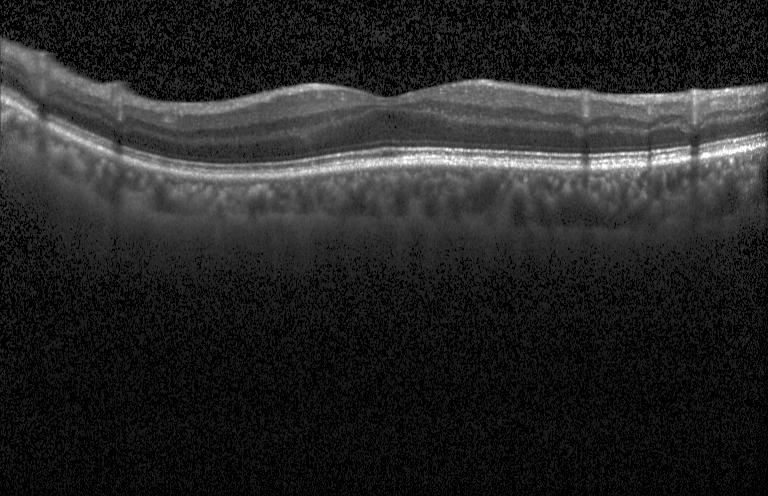

Dx: neither choroidal neovascularization, diabetic macular edema, nor drusen.